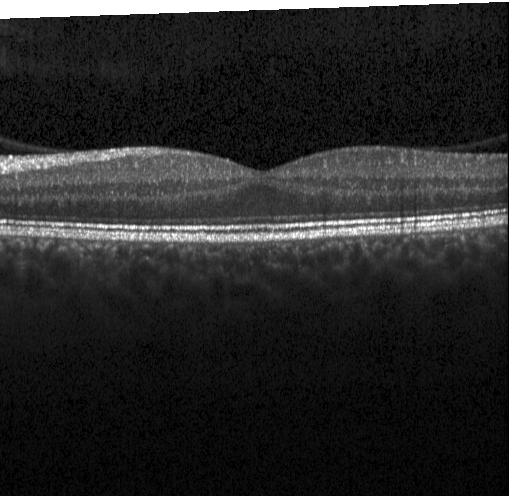
OCT line scan — Diagnosis: neither choroidal neovascularization, diabetic macular edema, nor drusen.